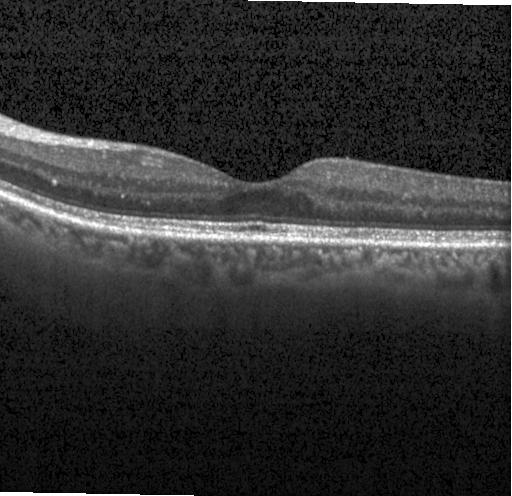 SD-OCT. Heidelberg Spectralis OCT system. OCT line scan
Diagnosis: neither CNV, DME, nor drusen.